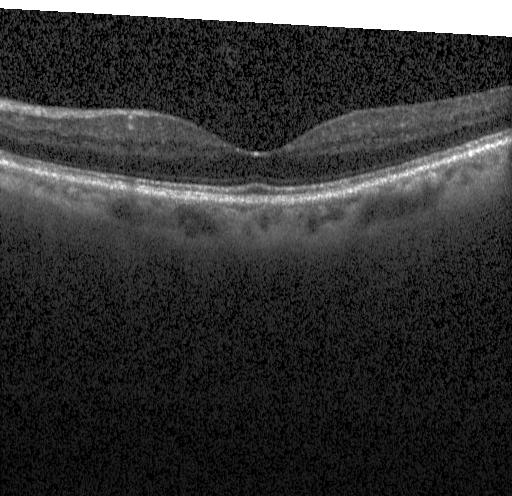
Optical coherence tomography scan
OCT finding: no evidence of choroidal neovascularization, diabetic macular edema, or drusen.